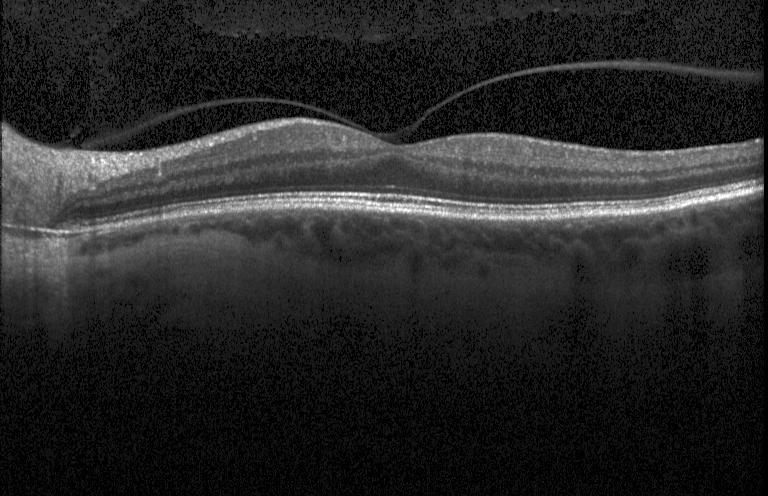

Assessment: neither choroidal neovascularization, diabetic macular edema, nor drusen.